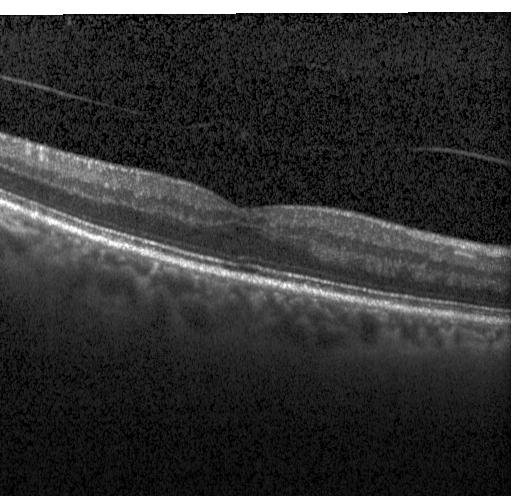

Diagnosis: neither choroidal neovascularization, diabetic macular edema, nor drusen.